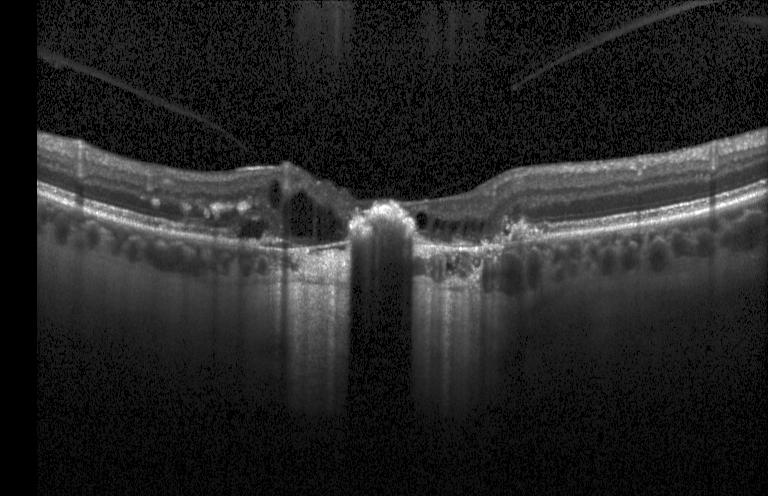 Retinal OCT cross-section showing choroidal neovascularization.